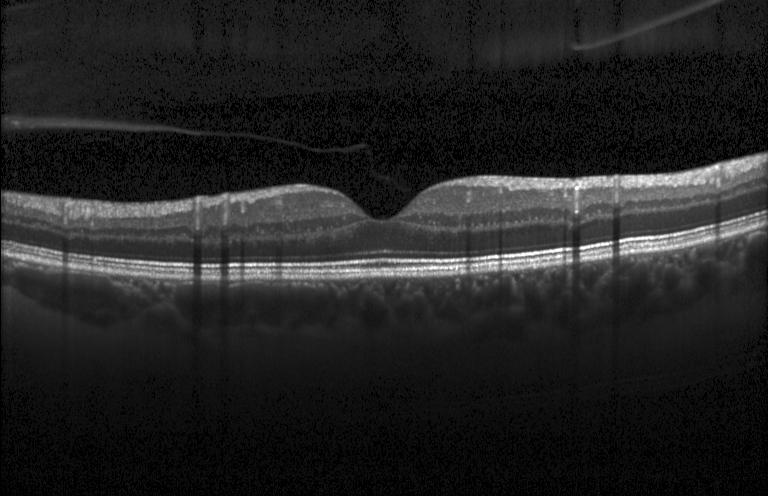

Macular OCT: no choroidal neovascularization, no diabetic macular edema, and no drusen.